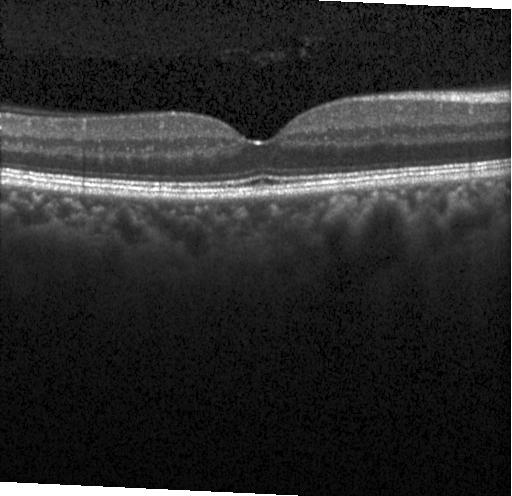
Finding: no CNV, no DME, and no drusen.